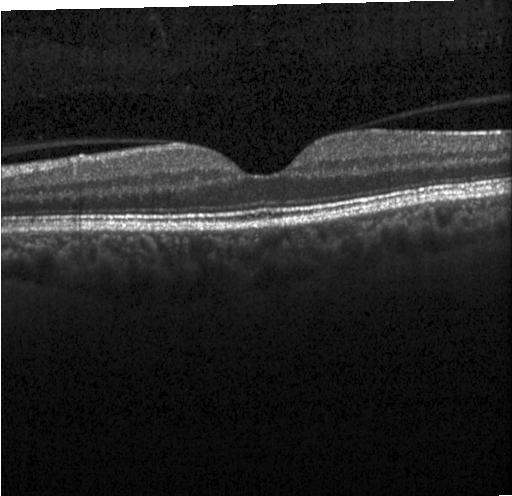 Finding: neither choroidal neovascularization, diabetic macular edema, nor drusen.